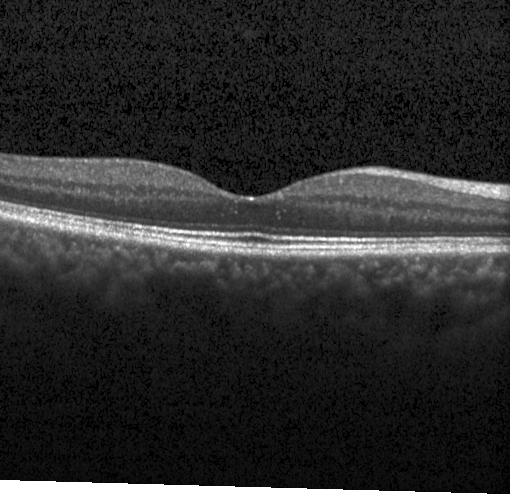
Finding: no choroidal neovascularization, diabetic macular edema, or drusen.